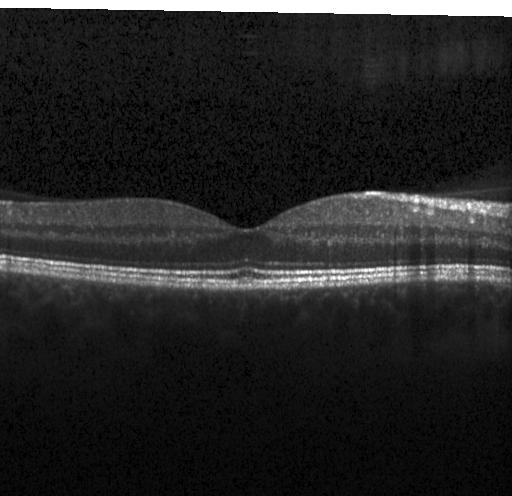 Horizontal scan through the fovea. OCT line scan. SD-OCT.
Impression: neither choroidal neovascularization, diabetic macular edema, nor drusen.